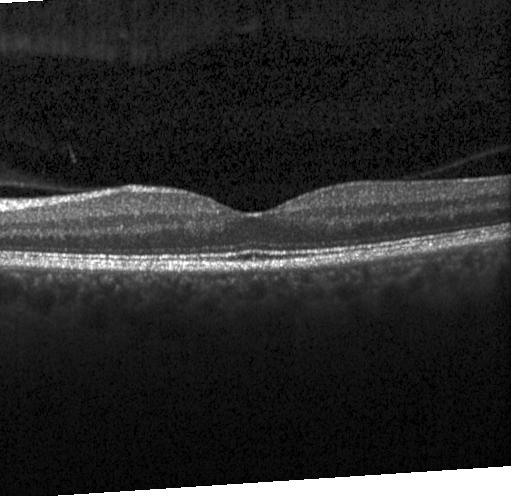 OCT B-scan. Spectral-domain OCT. Horizontal scan through the fovea.
Finding: neither choroidal neovascularization, diabetic macular edema, nor drusen.